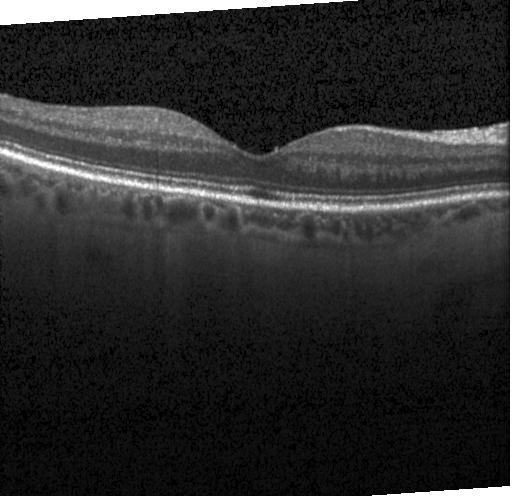

Macular scan · optical coherence tomography scan. The scan shows neither choroidal neovascularization, diabetic macular edema, nor drusen.